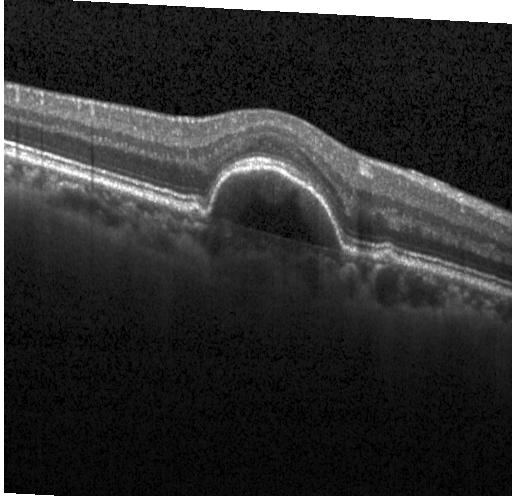
Macular scan, Heidelberg Spectralis OCT system, OCT B-scan — Impression: a choroidal neovascular membrane.